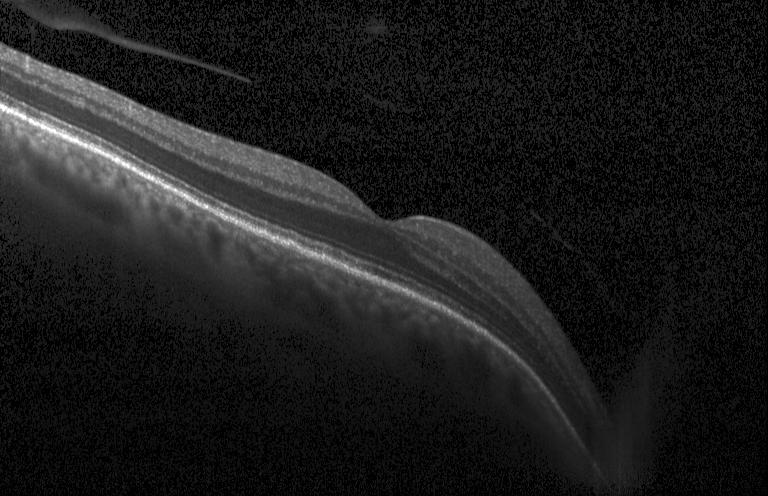

Diagnosis: no CNV, no DME, and no drusen.